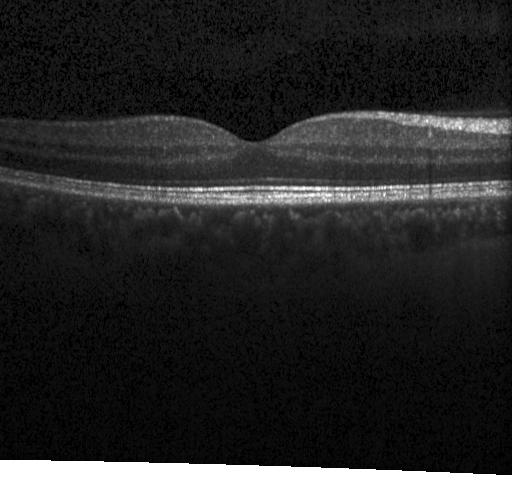

Spectral-domain OCT, OCT B-scan, horizontal scan through the fovea. Diagnosis: no CNV, DME, or drusen.